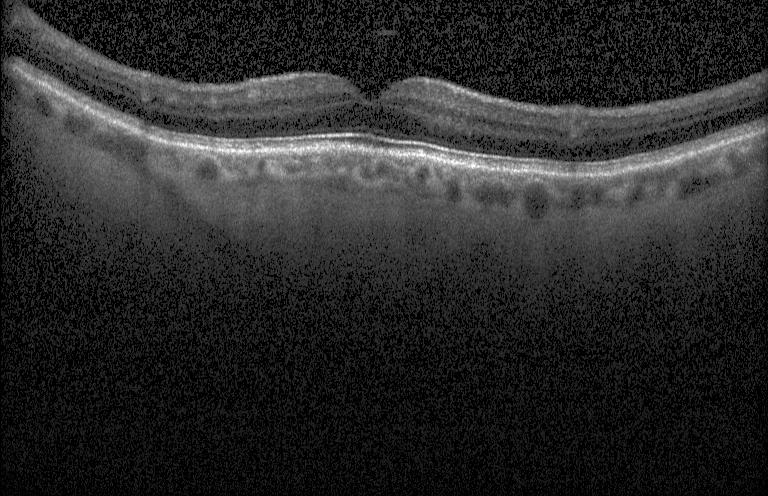 OCT B-scan, through the macula.
Impression: no evidence of choroidal neovascularization, diabetic macular edema, or drusen.